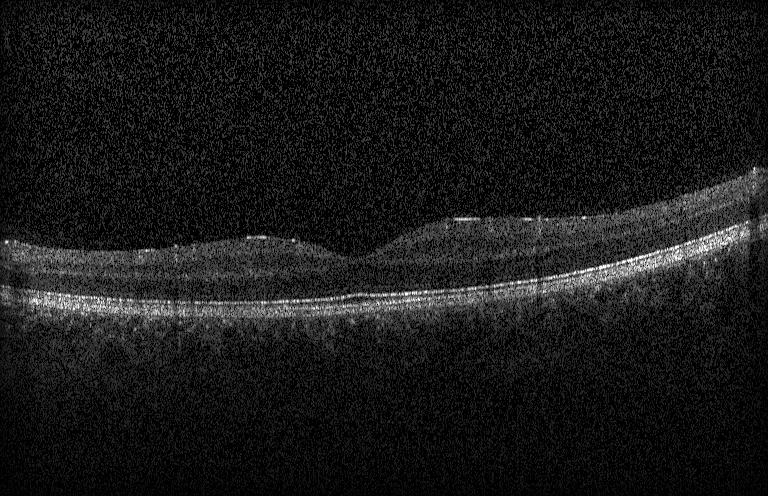 Spectral-domain OCT · Heidelberg Spectralis OCT system · horizontal scan through the fovea · optical coherence tomography scan. Diagnosis: neither choroidal neovascularization, diabetic macular edema, nor drusen.